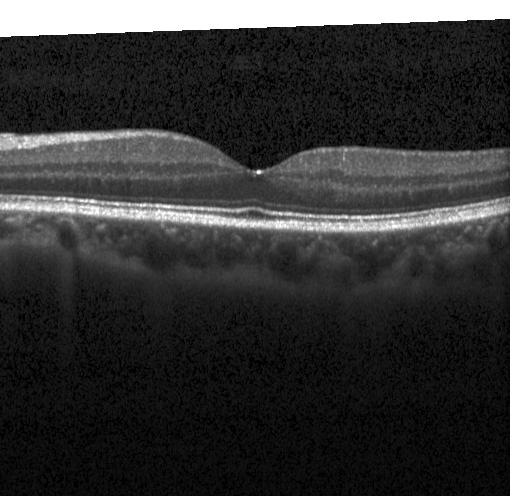 Macular OCT: no choroidal neovascularization, no diabetic macular edema, and no drusen.